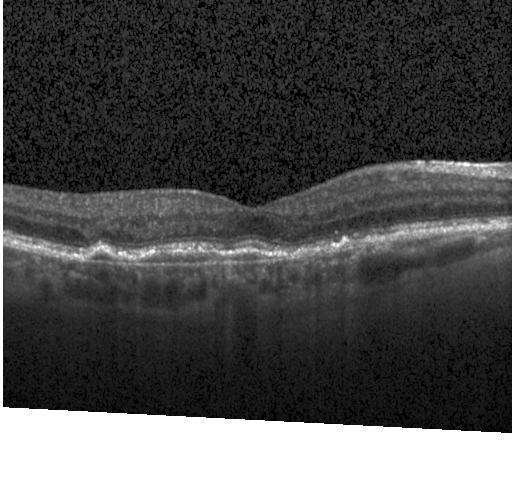
Dx: a choroidal neovascular membrane.